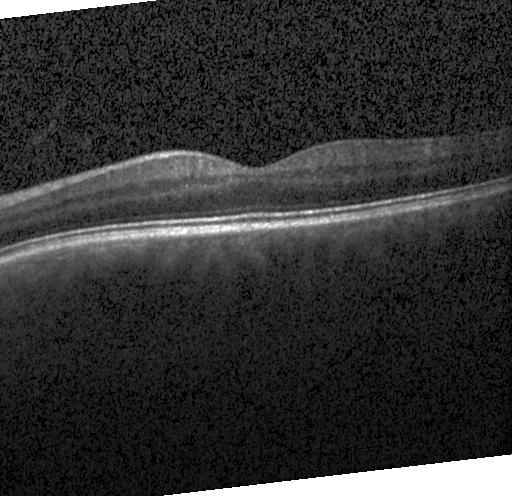

Dx: no choroidal neovascularization, no diabetic macular edema, and no drusen.